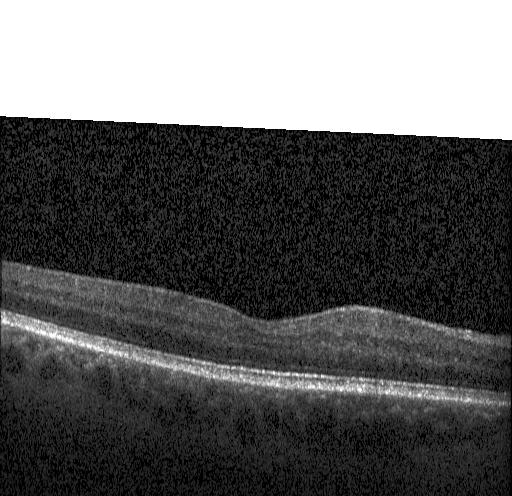
Instrument: Heidelberg Spectralis, macular scan, OCT B-scan. Assessment: no choroidal neovascularization, no diabetic macular edema, and no drusen.